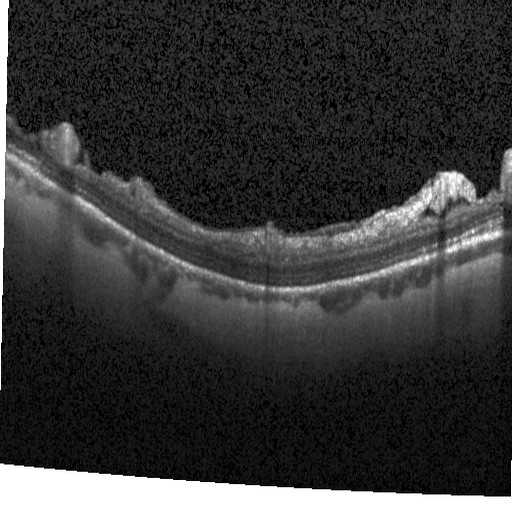
The scan shows diabetic macular edema.